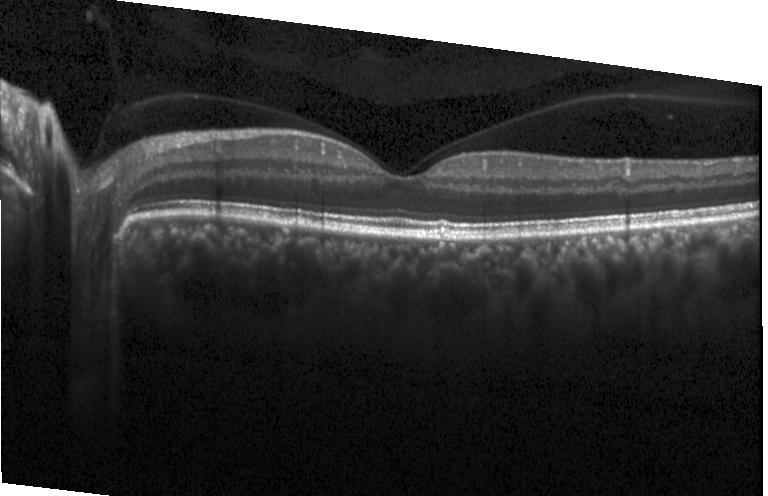
Macular scan; optical coherence tomography B-scan
OCT finding: multiple drusen.